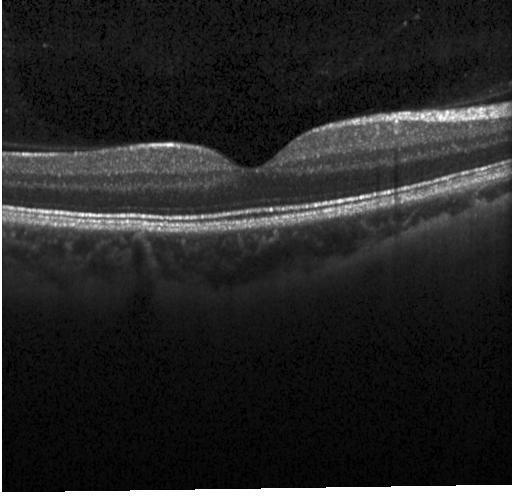 Acquired on a Heidelberg Spectralis · spectral-domain optical coherence tomography · through the macula · retinal OCT B-scan — Neither CNV, DME, nor drusen.